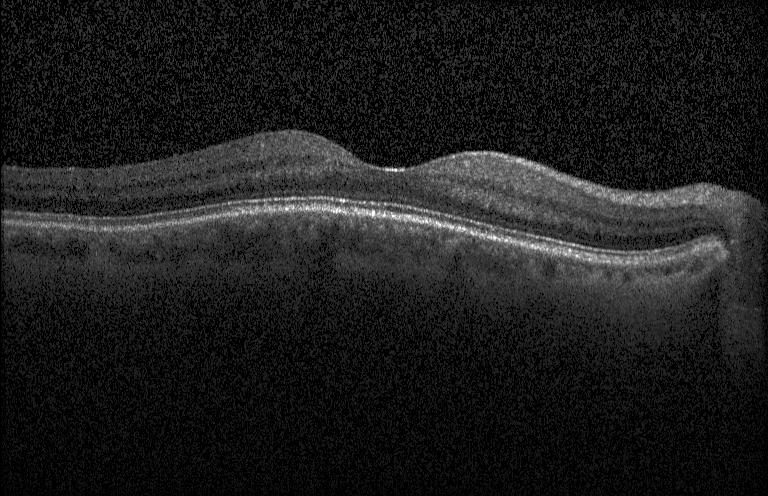
Heidelberg Spectralis OCT system · optical coherence tomography B-scan — The scan shows no choroidal neovascularization, diabetic macular edema, or drusen.